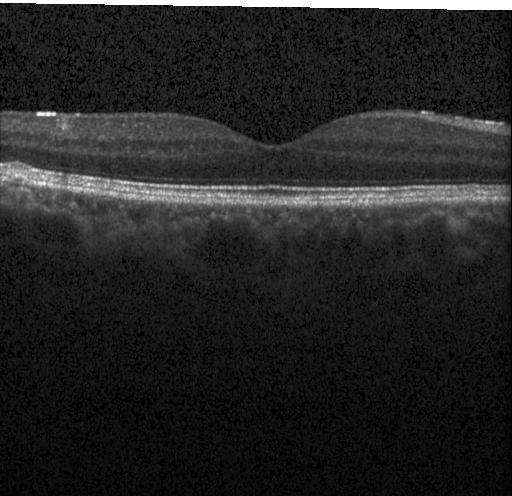
Optical coherence tomography scan · horizontal scan through the fovea — OCT finding: neither choroidal neovascularization, diabetic macular edema, nor drusen.